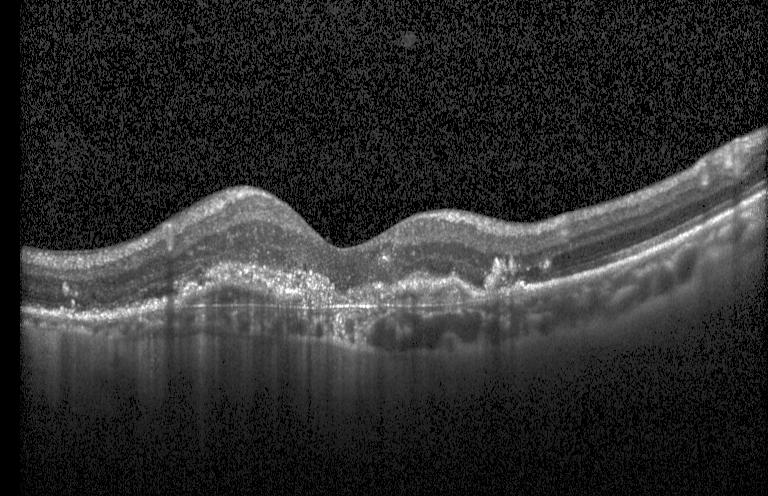

Heidelberg Spectralis OCT system; optical coherence tomography B-scan.
A choroidal neovascular membrane.